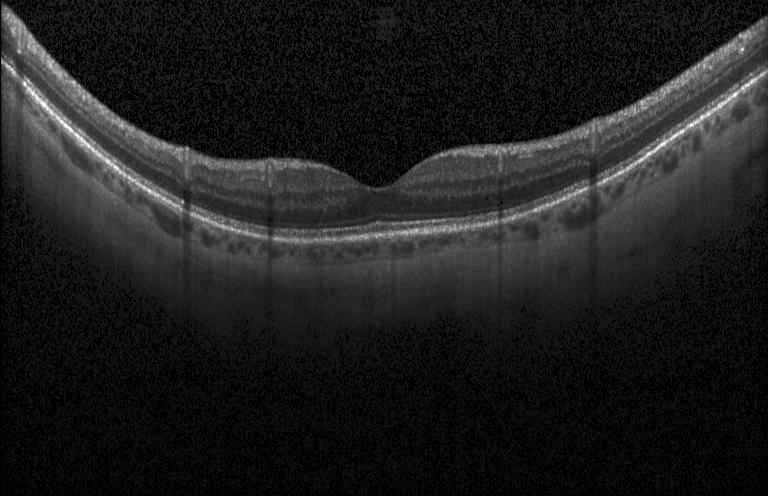
Retinal OCT cross-section.
Dx: no choroidal neovascularization, no diabetic macular edema, and no drusen.